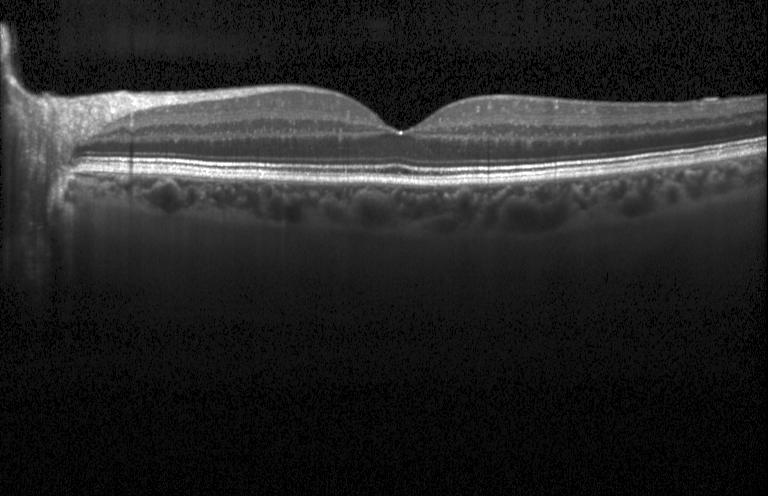
Diagnosis: no choroidal neovascularization, diabetic macular edema, or drusen.